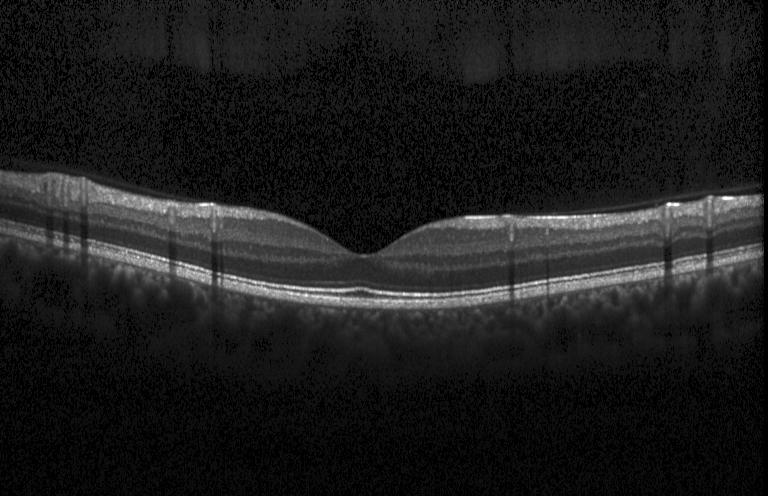
Spectral-domain OCT; acquired on a Heidelberg Spectralis; OCT B-scan; fovea-centered
The scan shows no CNV, DME, or drusen.